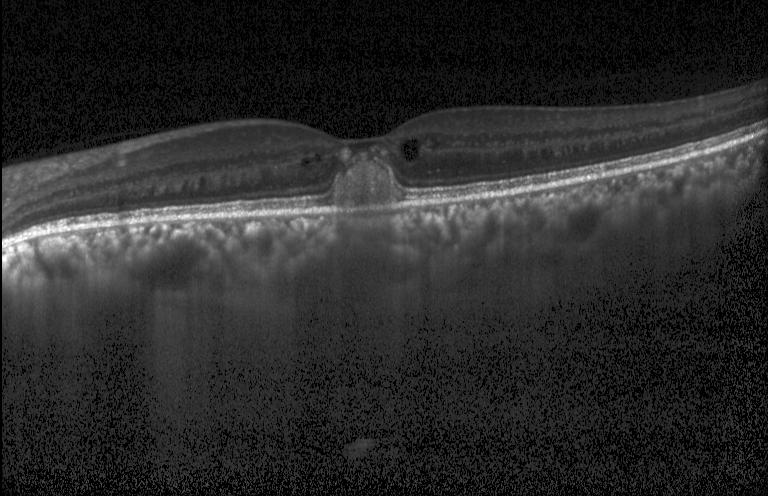

OCT finding: CNV.